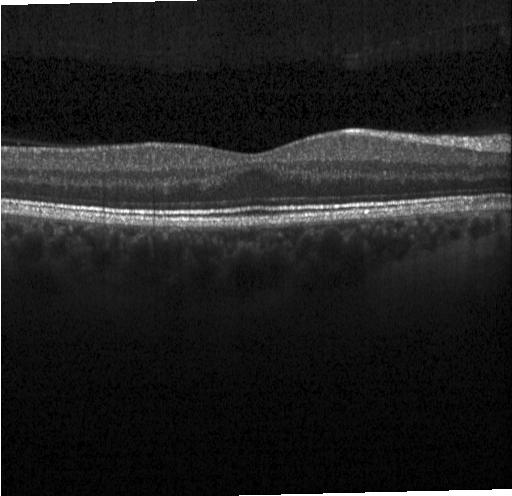 Retinal OCT B-scan. OCT finding: no CNV, no DME, and no drusen.